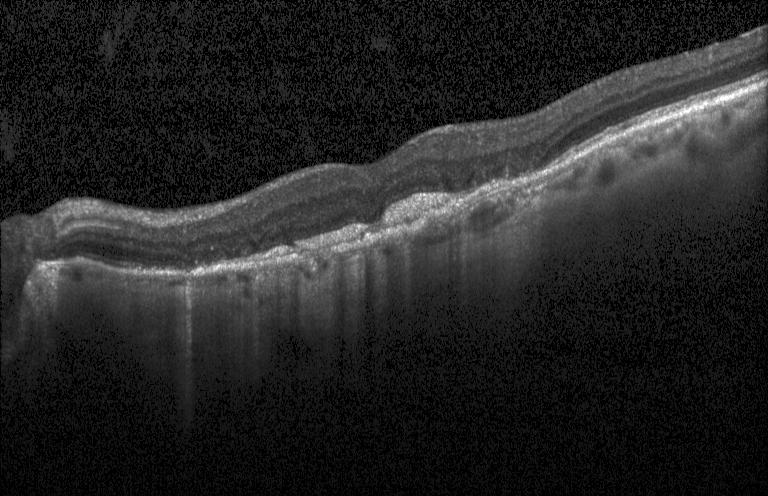 Macular OCT: CNV.